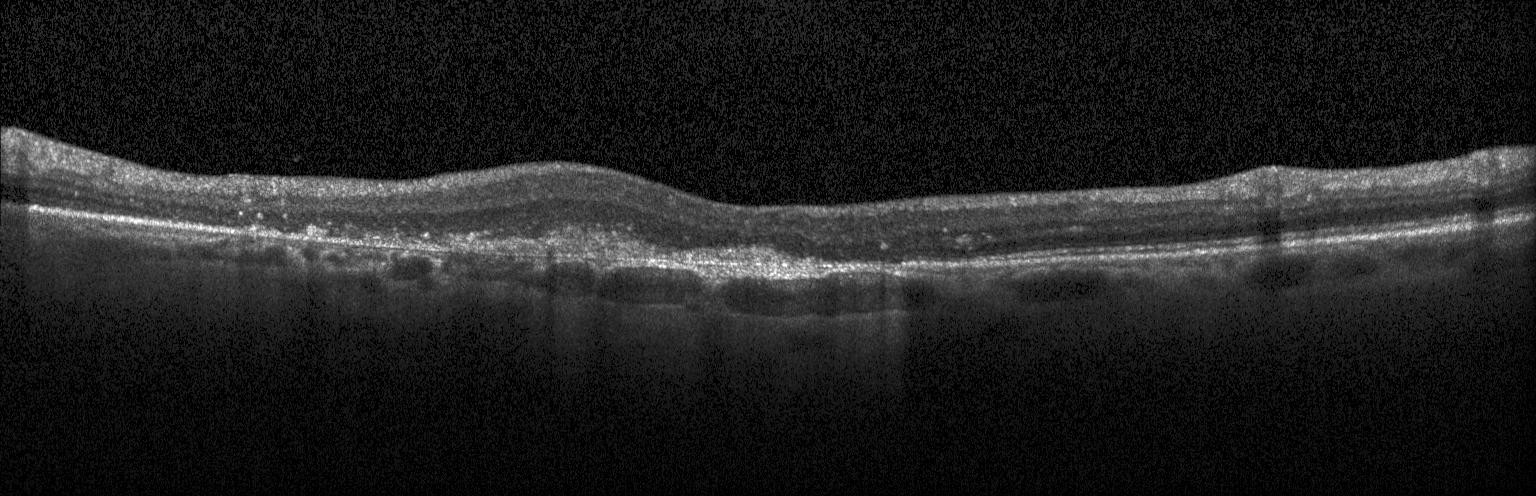

Optical coherence tomography B-scan · instrument: Heidelberg Spectralis · macular scan · spectral-domain OCT
Diagnosis: a choroidal neovascular membrane.